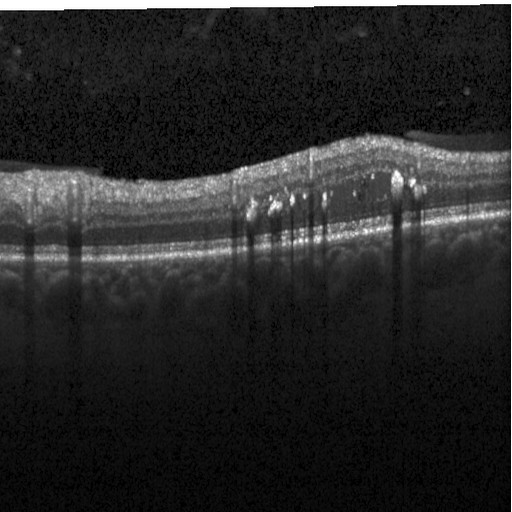
OCT B-scan. Centered on the fovea
Diabetic macular edema (DME).